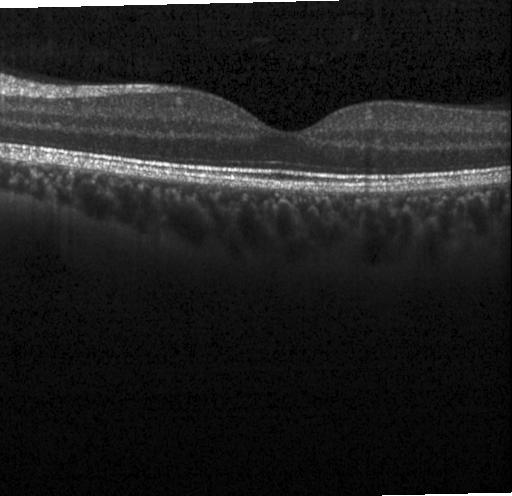
OCT line scan · macular scan. No evidence of CNV, DME, or drusen.